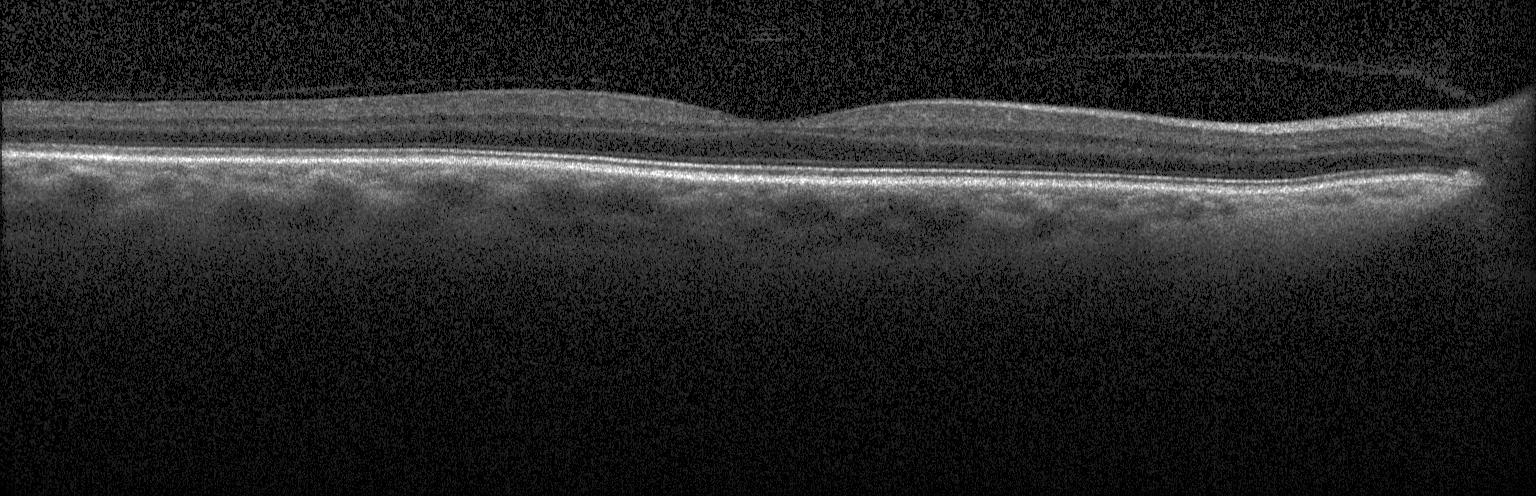

Dx: no CNV, DME, or drusen.